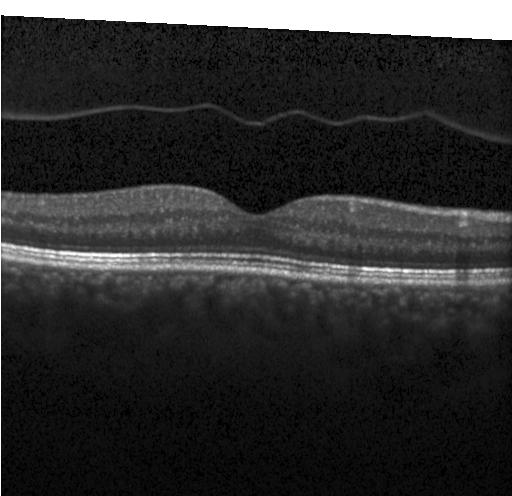 Optical coherence tomography B-scan. Spectral-domain OCT. Heidelberg Spectralis OCT system. Through the macula. Diagnosis: no evidence of CNV, DME, or drusen.